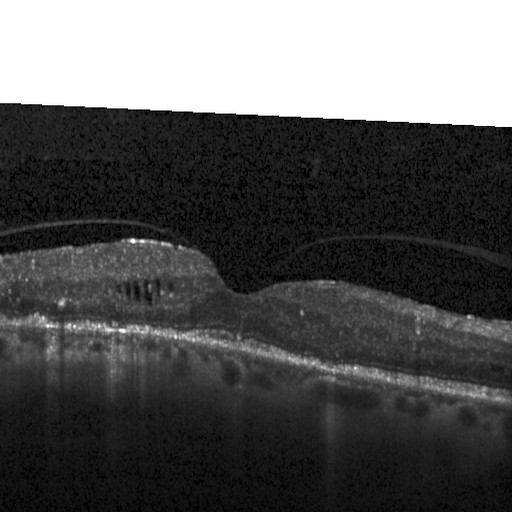 OCT scan showing DME.